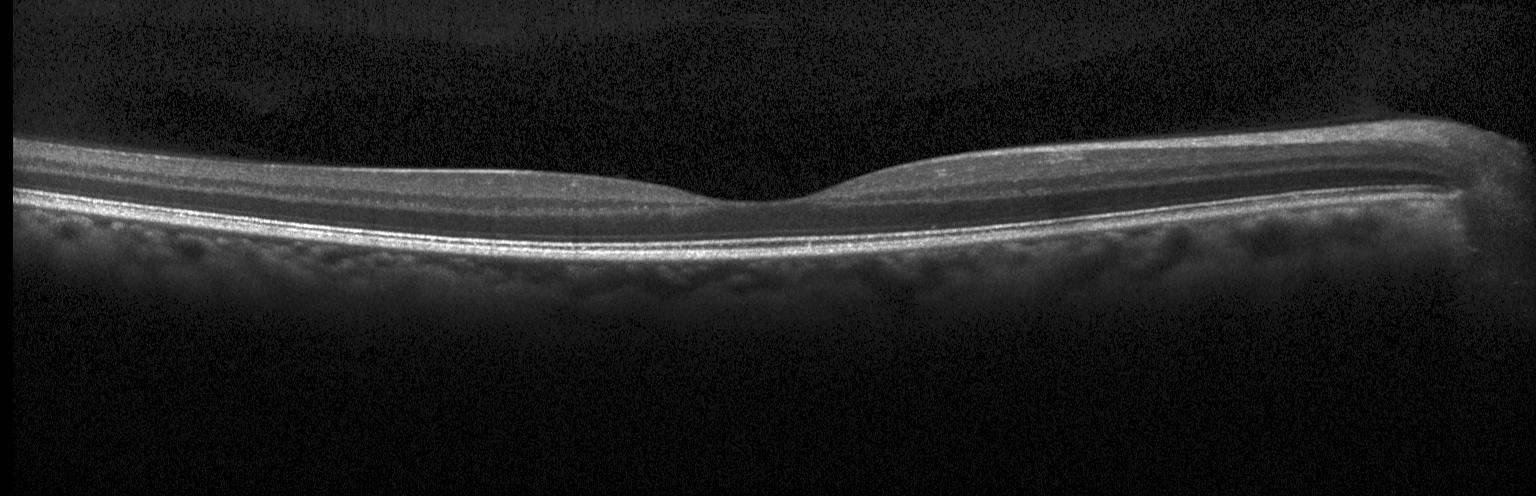 Impression: no evidence of choroidal neovascularization, diabetic macular edema, or drusen.